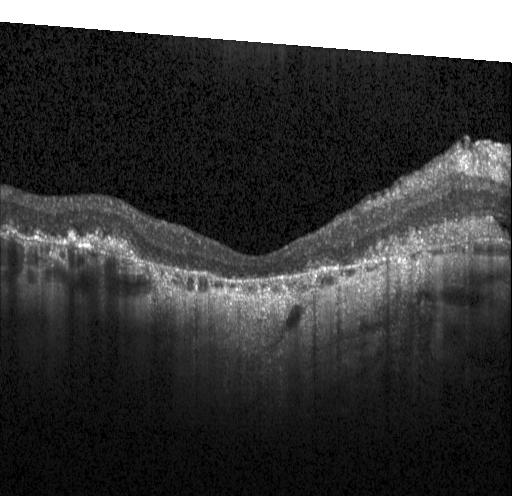 Through the macula. SD-OCT. OCT line scan — Diagnosis: a choroidal neovascular membrane.